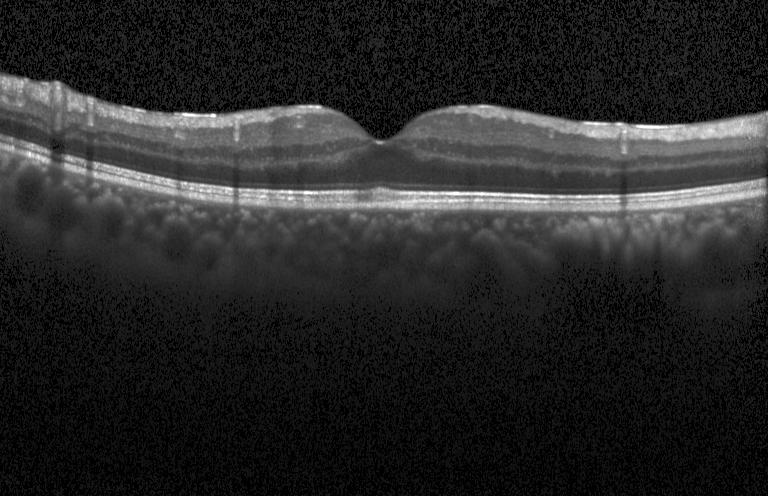 Dx: no CNV, no DME, and no drusen.